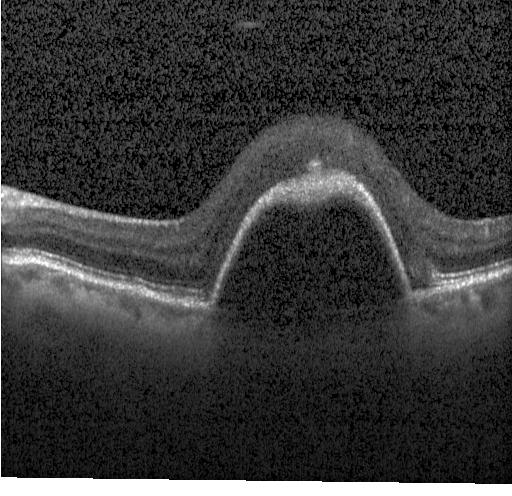
Optical coherence tomography scan, spectral-domain OCT, fovea-centered. Assessment: choroidal neovascularization.